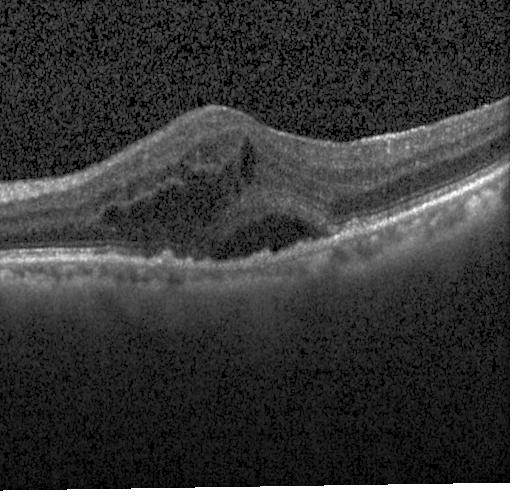

Impression: diabetic macular edema (DME).